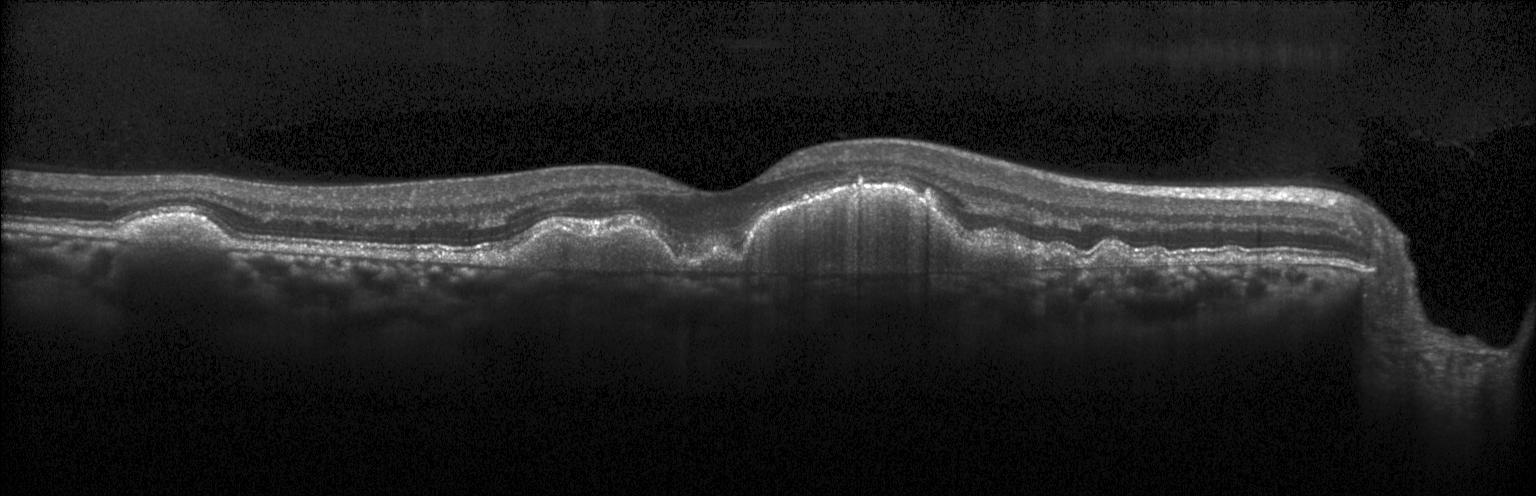 Macular OCT: sub-RPE drusenoid deposits.